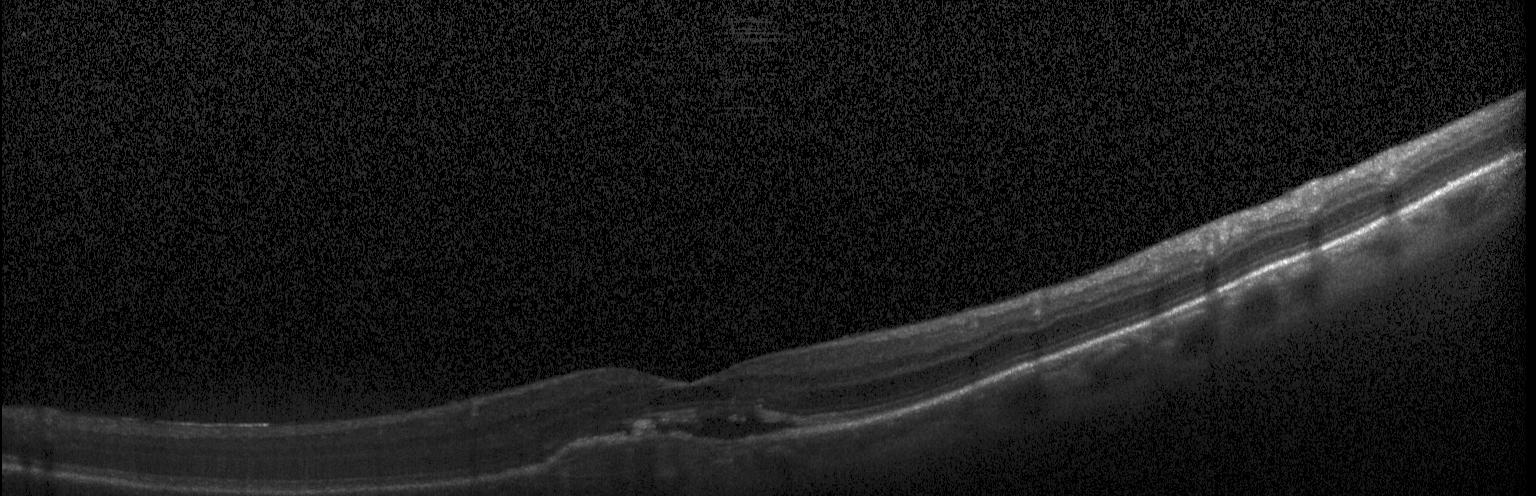
Impression: choroidal neovascularization.